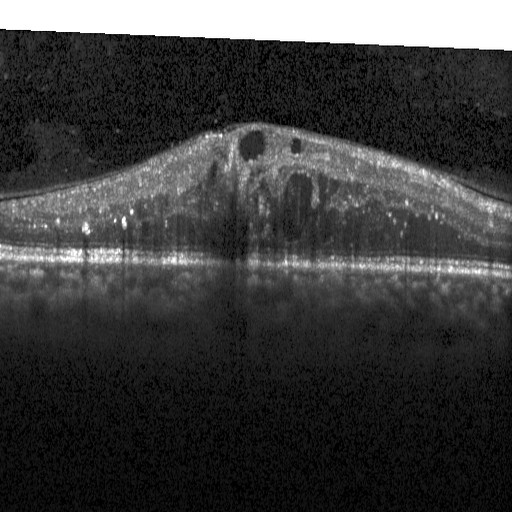 OCT line scan. Heidelberg Spectralis. Spectral-domain OCT. Centered on the fovea.
Dx: diabetic macular edema (DME).